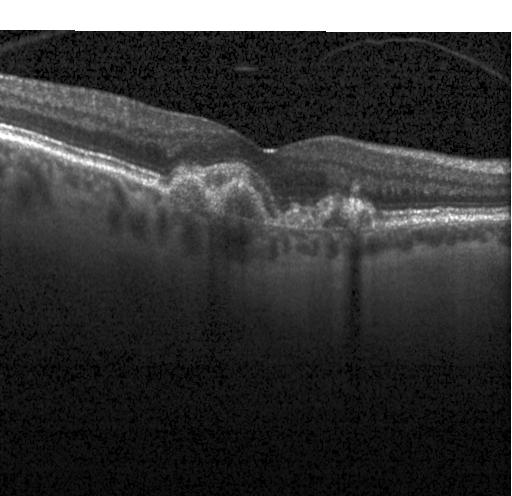

OCT B-scan. Finding: a choroidal neovascular membrane.